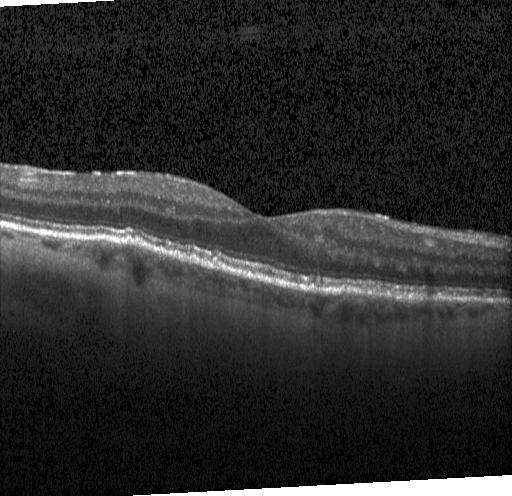

Diagnosis: multiple drusen.